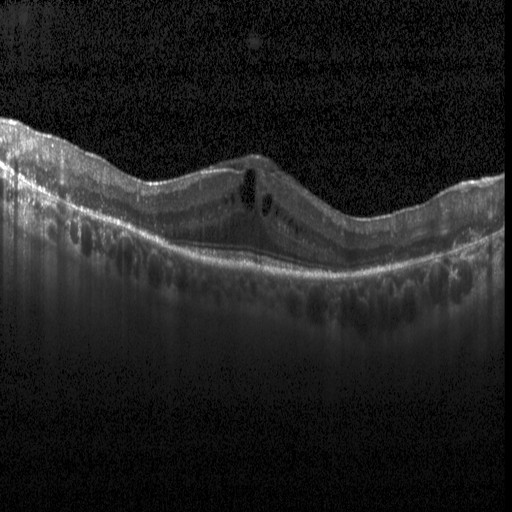 Optical coherence tomography scan
Diagnosis: diabetic macular edema (DME).